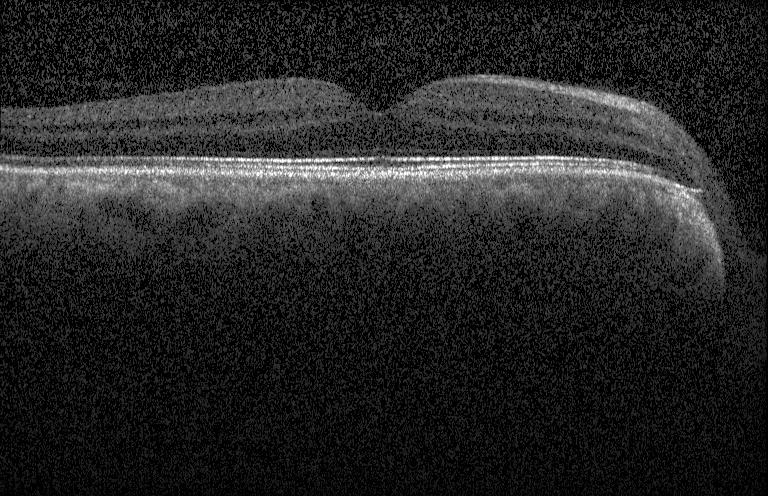

OCT B-scan — This B-scan demonstrates no choroidal neovascularization, no diabetic macular edema, and no drusen.